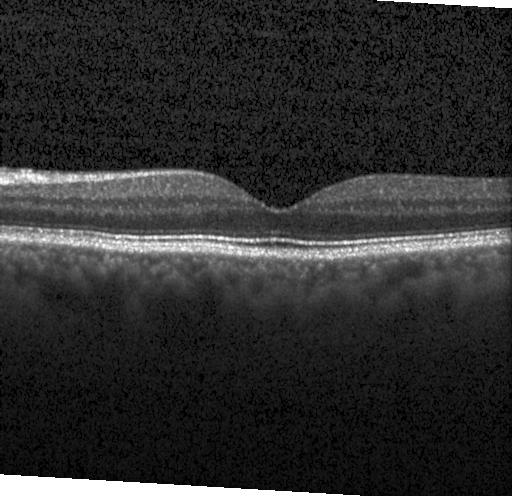

Spectral-domain optical coherence tomography. Heidelberg Spectralis. Optical coherence tomography scan. Centered on the fovea.
Finding: no choroidal neovascularization, diabetic macular edema, or drusen.